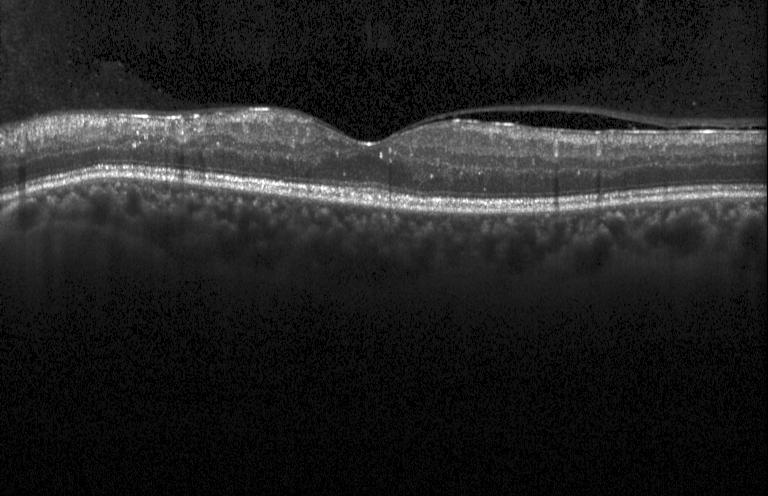

Macular scan, Heidelberg Spectralis OCT system, SD-OCT, optical coherence tomography B-scan. Diagnosis: diabetic macular edema (DME).